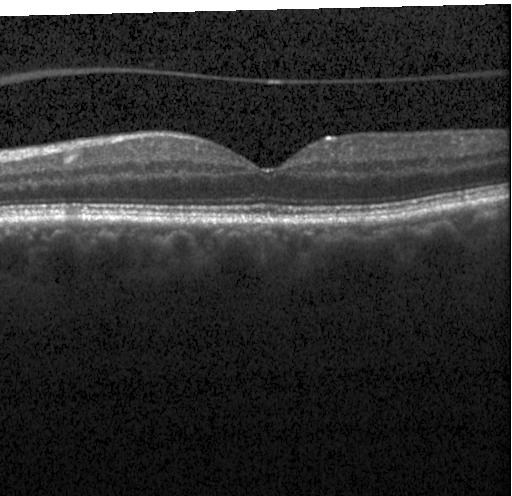
OCT B-scan showing no evidence of choroidal neovascularization, diabetic macular edema, or drusen.